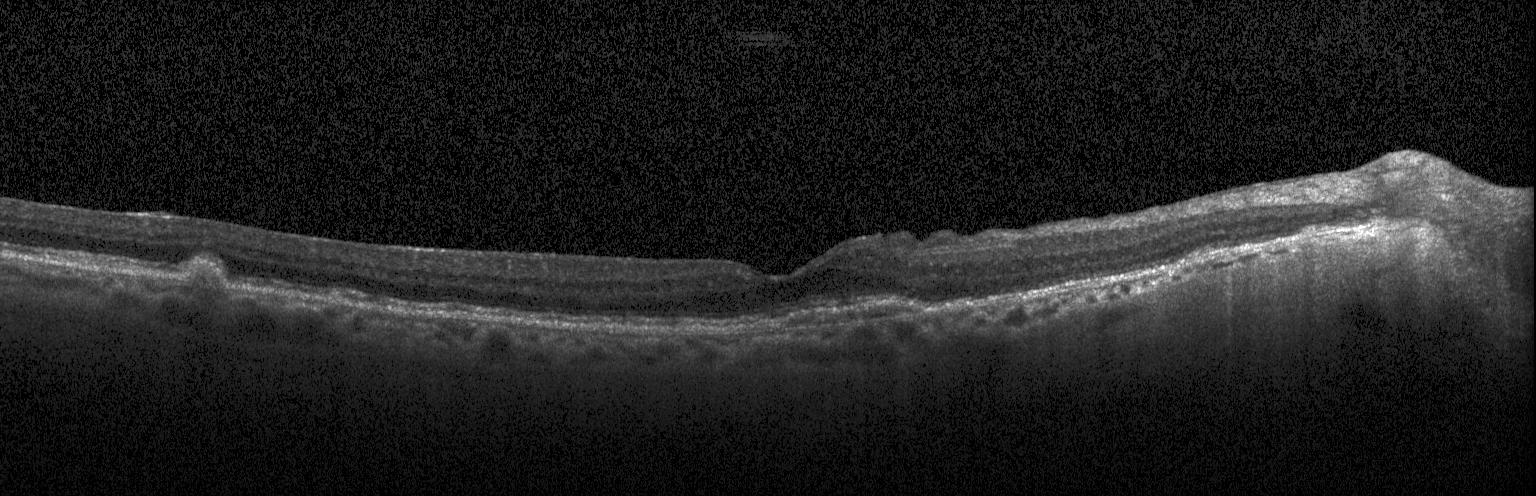 Optical coherence tomography B-scan · fovea-centered · SD-OCT
The scan shows CNV.